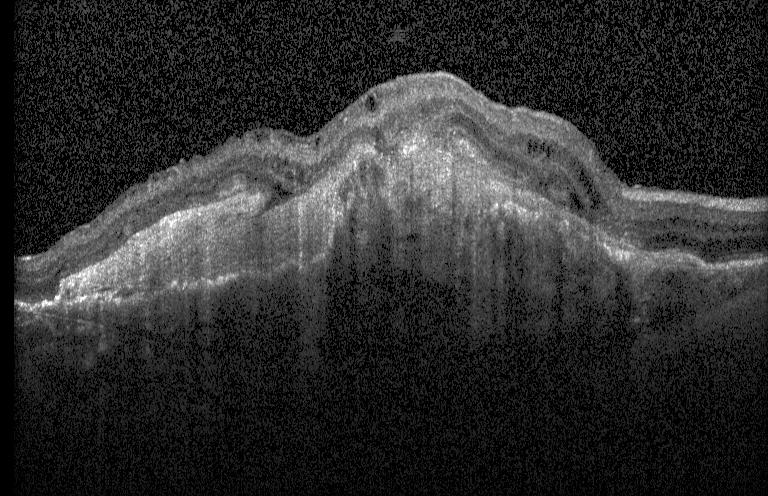
SD-OCT, retinal OCT B-scan, horizontal scan through the fovea.
OCT finding: a choroidal neovascular membrane.